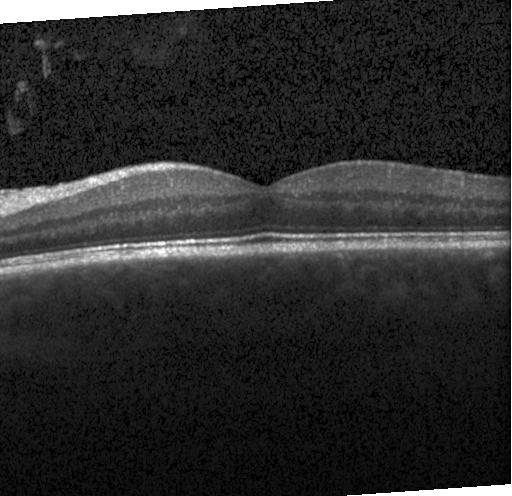 OCT scan showing neither choroidal neovascularization, diabetic macular edema, nor drusen.